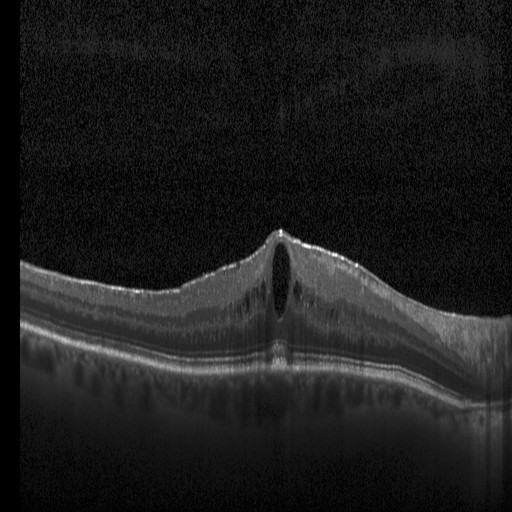 Acquired on a Heidelberg Spectralis, retinal OCT cross-section, SD-OCT.
Finding: diabetic macular edema (DME).